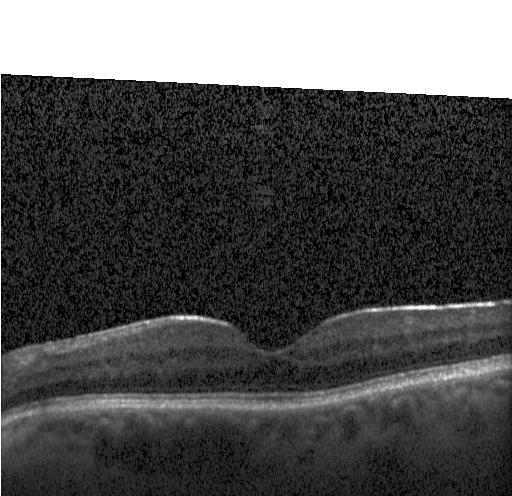

Optical coherence tomography scan, through the macula, SD-OCT, instrument: Heidelberg Spectralis. Diagnosis: no choroidal neovascularization, diabetic macular edema, or drusen.